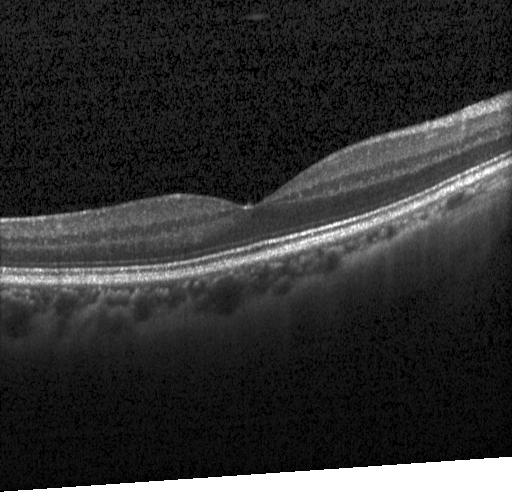 OCT B-scan; spectral-domain optical coherence tomography; fovea-centered. No choroidal neovascularization, diabetic macular edema, or drusen.